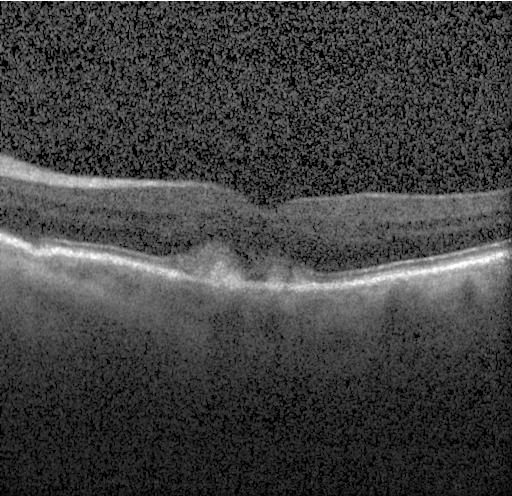 Retinal OCT B-scan — Macular OCT: choroidal neovascularization (CNV).